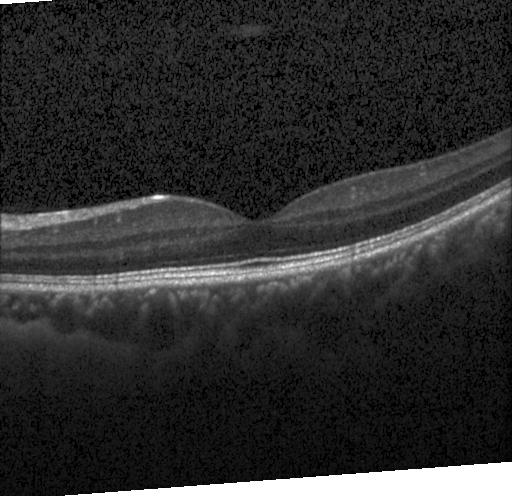

Spectral-domain OCT; macular scan; OCT line scan.
Dx: no choroidal neovascularization, no diabetic macular edema, and no drusen.